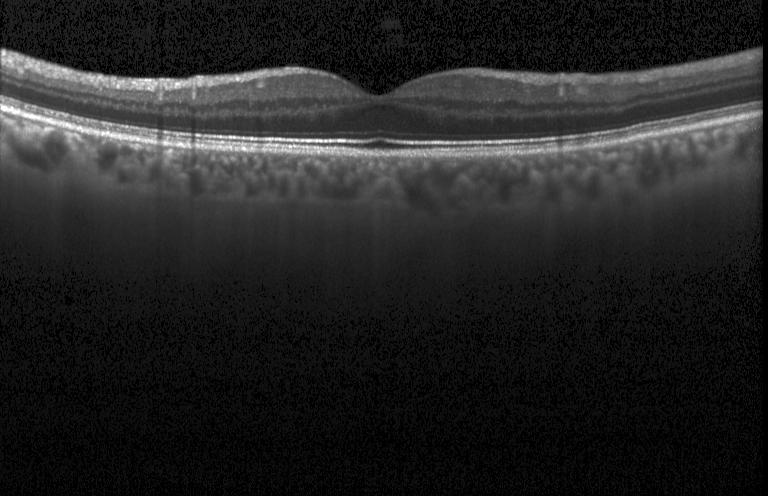
OCT B-scan showing no choroidal neovascularization, no diabetic macular edema, and no drusen.